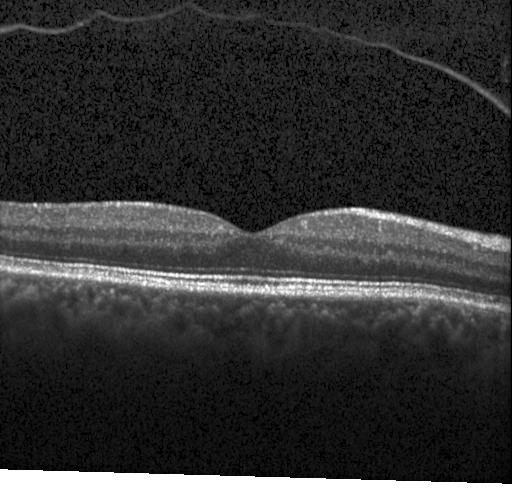
OCT line scan
Impression: no evidence of choroidal neovascularization, diabetic macular edema, or drusen.